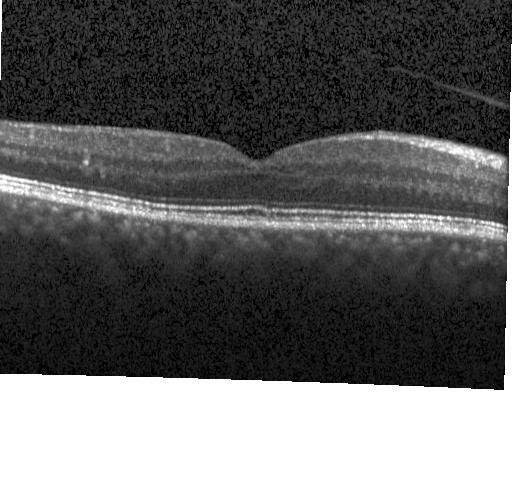
Macular OCT demonstrating no choroidal neovascularization, no diabetic macular edema, and no drusen.